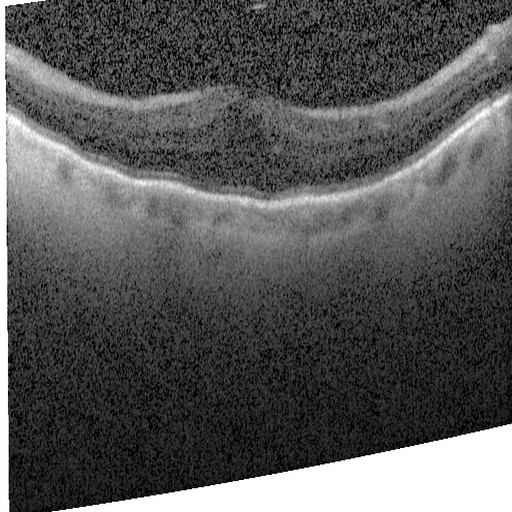

Macular OCT: diabetic macular edema.